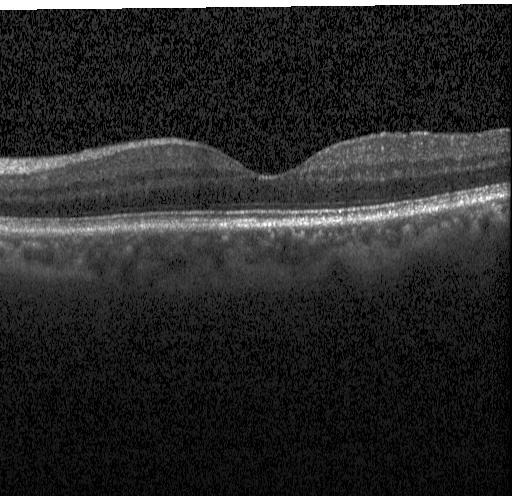
Impression: no evidence of CNV, DME, or drusen.